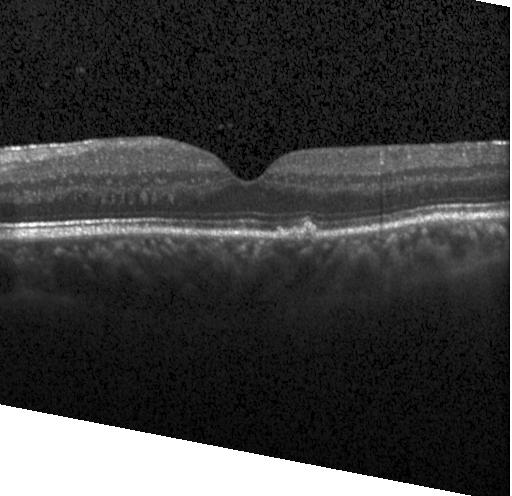
Optical coherence tomography B-scan
Assessment: sub-RPE drusenoid deposits.